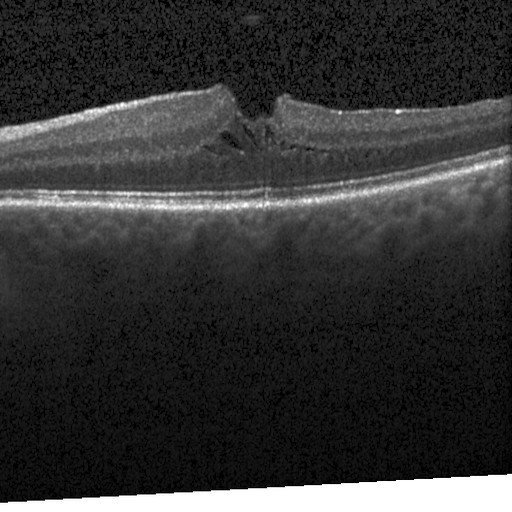

Macular OCT demonstrating DME.